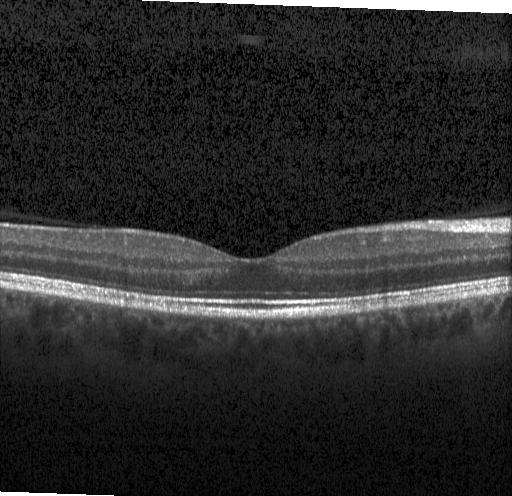 OCT line scan. The scan shows no CNV, no DME, and no drusen.